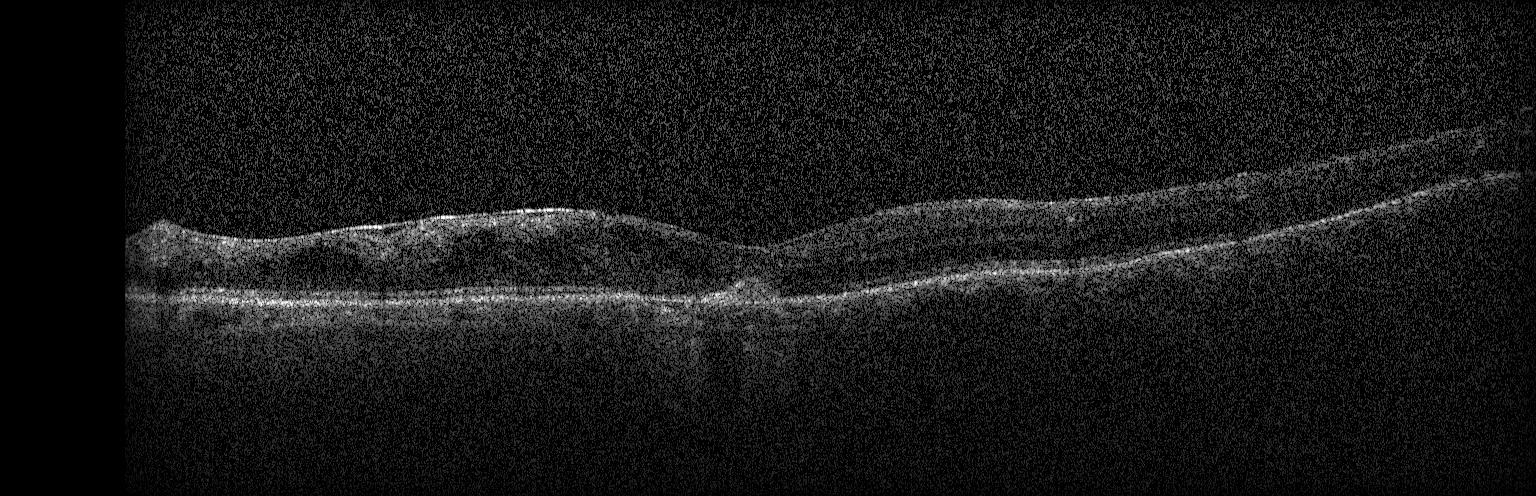
Horizontal scan through the fovea; spectral-domain OCT; retinal OCT cross-section; acquired on a Heidelberg Spectralis — The scan shows choroidal neovascularization.